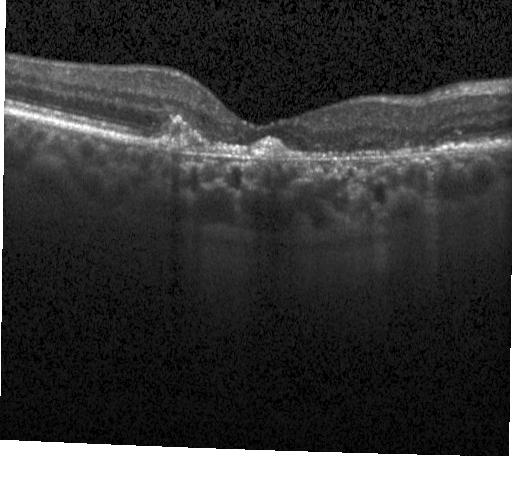
OCT line scan · macular scan · Heidelberg Spectralis.
Diagnosis: choroidal neovascularization (CNV).